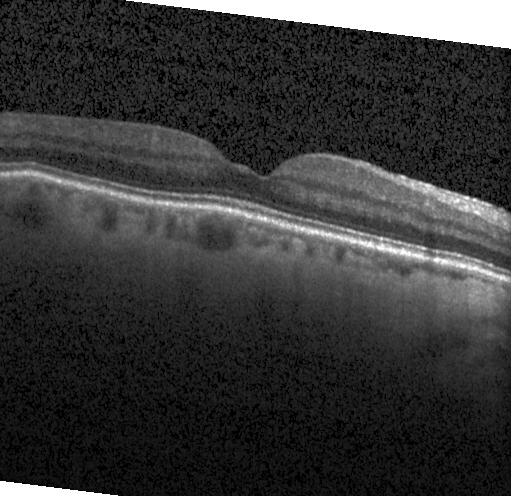 Optical coherence tomography scan. Impression: no evidence of choroidal neovascularization, diabetic macular edema, or drusen.